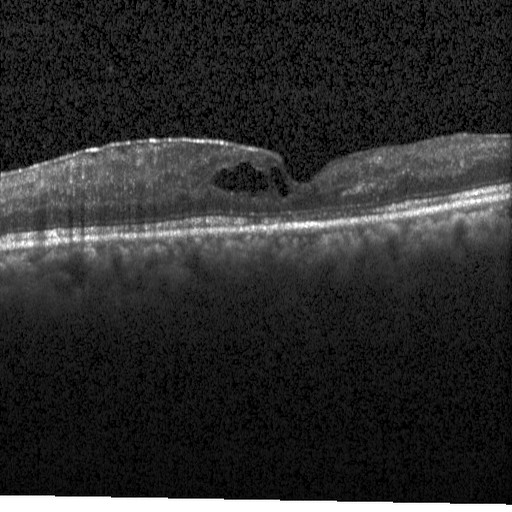 Centered on the fovea; retinal OCT cross-section; spectral-domain OCT; Heidelberg Spectralis OCT system. Diagnosis: diabetic macular edema (DME).